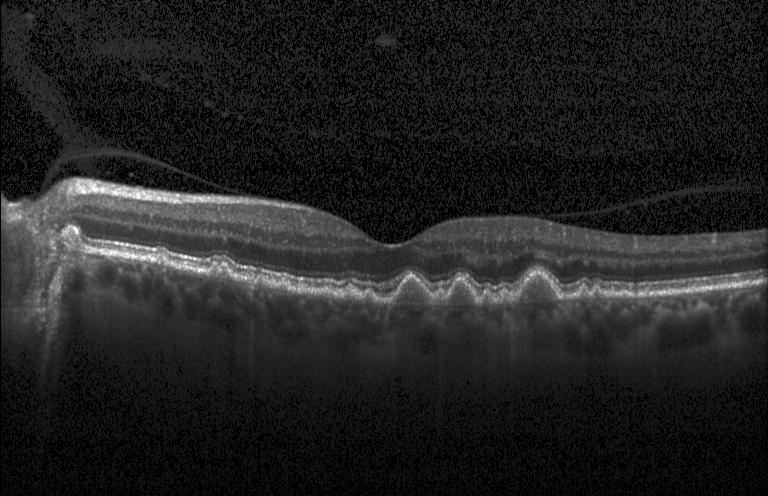
Impression: multiple drusen.